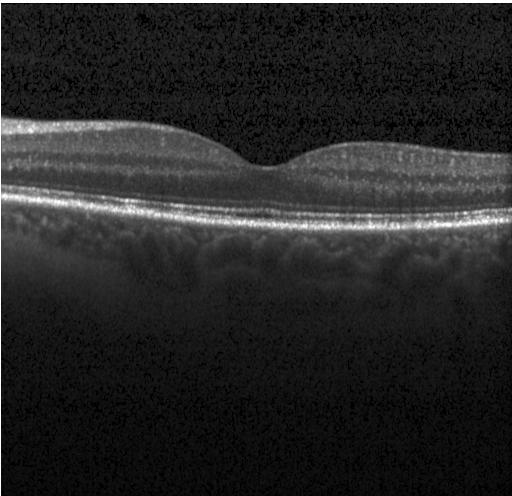 This B-scan demonstrates no choroidal neovascularization, no diabetic macular edema, and no drusen.